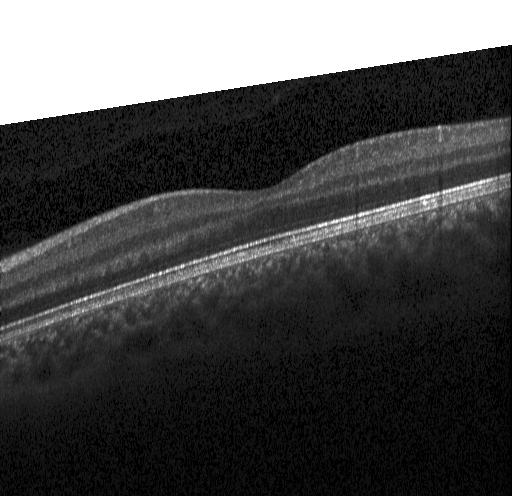 Macular OCT: neither choroidal neovascularization, diabetic macular edema, nor drusen.